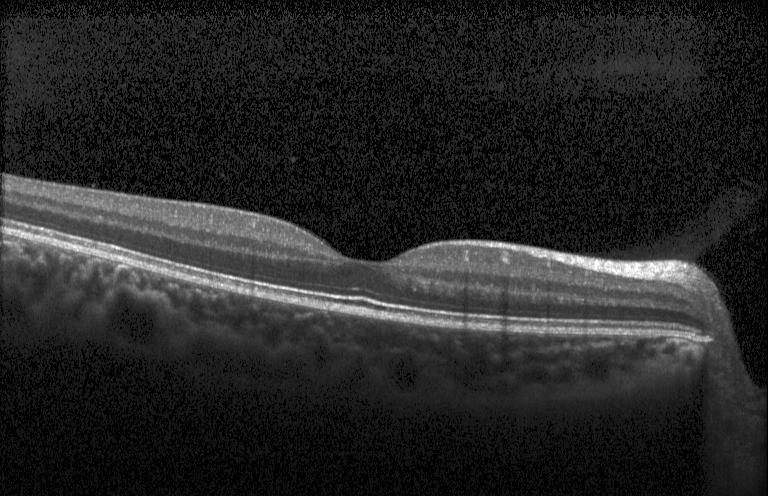

SD-OCT · retinal OCT cross-section · Heidelberg Spectralis OCT system. OCT finding: neither choroidal neovascularization, diabetic macular edema, nor drusen.